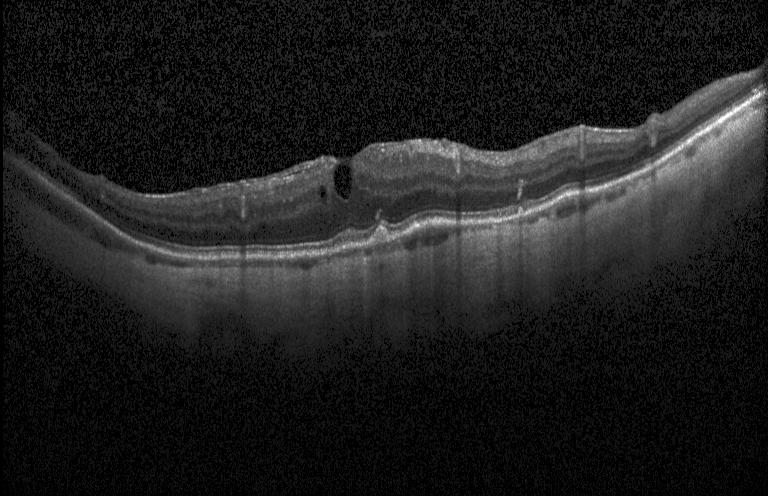

OCT line scan, instrument: Heidelberg Spectralis
Finding: drusen.